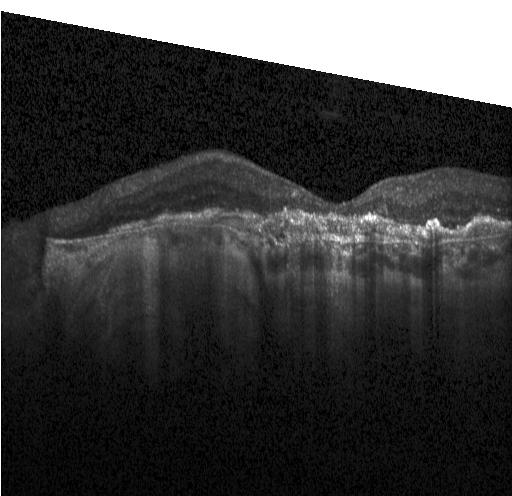 The scan shows choroidal neovascularization (CNV).